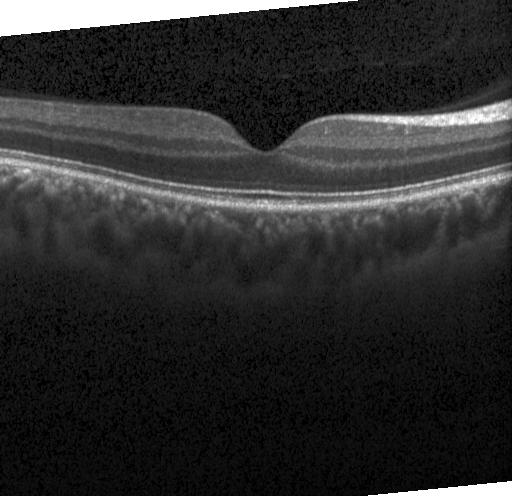 Diagnosis: no choroidal neovascularization, no diabetic macular edema, and no drusen.